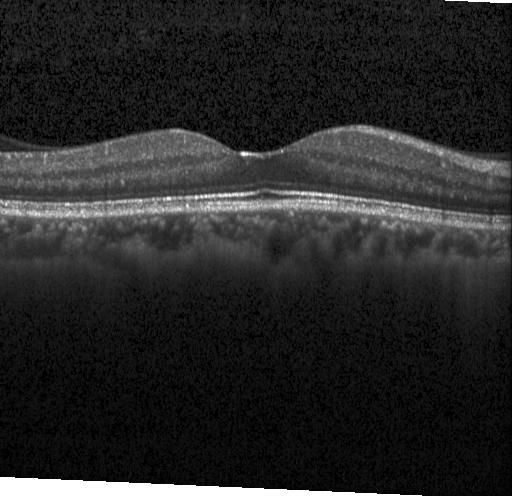
Spectral-domain optical coherence tomography; Heidelberg Spectralis OCT system; optical coherence tomography scan. Diagnosis: no CNV, no DME, and no drusen.